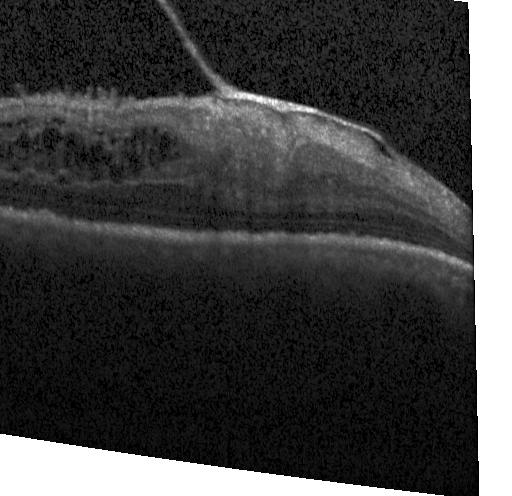
Impression: diabetic macular edema (DME).